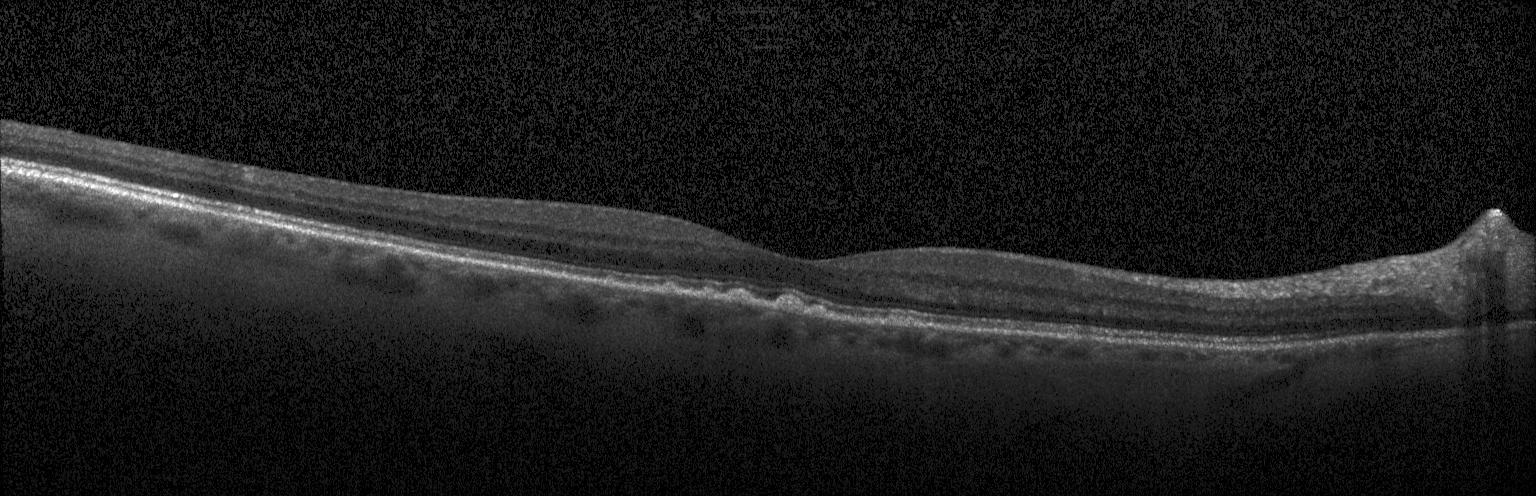
Impression: drusen.